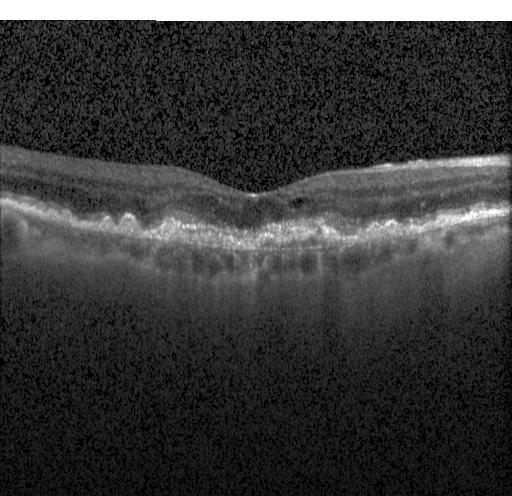 Spectral-domain OCT · OCT line scan · horizontal scan through the fovea · instrument: Heidelberg Spectralis — The scan shows a choroidal neovascular membrane.